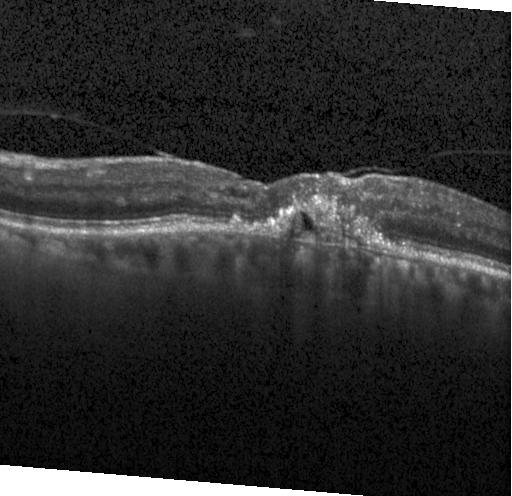

Acquired on a Heidelberg Spectralis. Retinal OCT B-scan. Macular scan. Spectral-domain OCT
The scan shows a choroidal neovascular membrane.